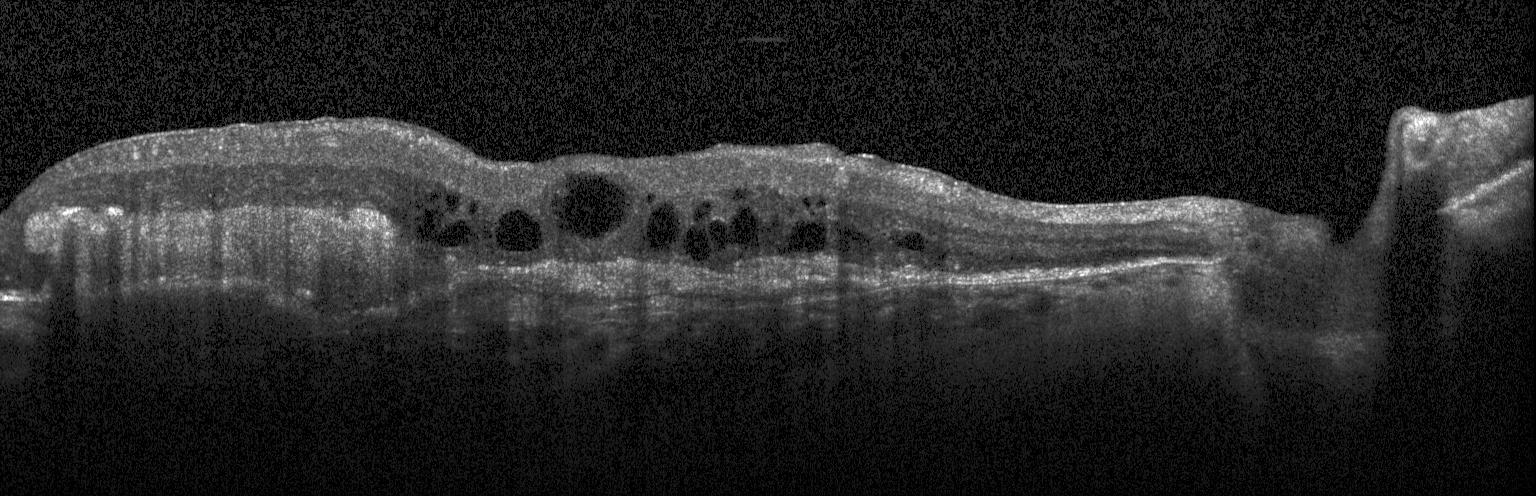

Retinal OCT cross-section, Heidelberg Spectralis OCT system — Diagnosis: a choroidal neovascular membrane.